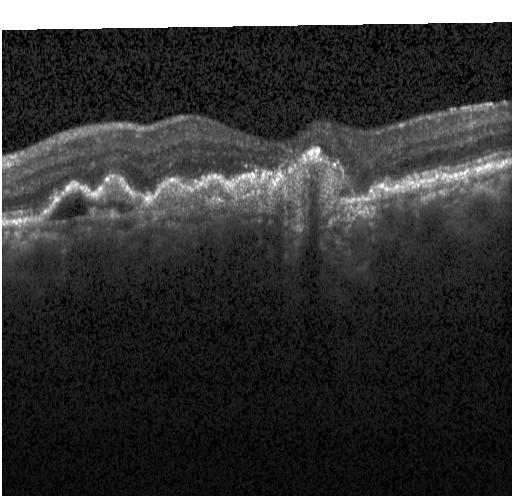
Dx: CNV.